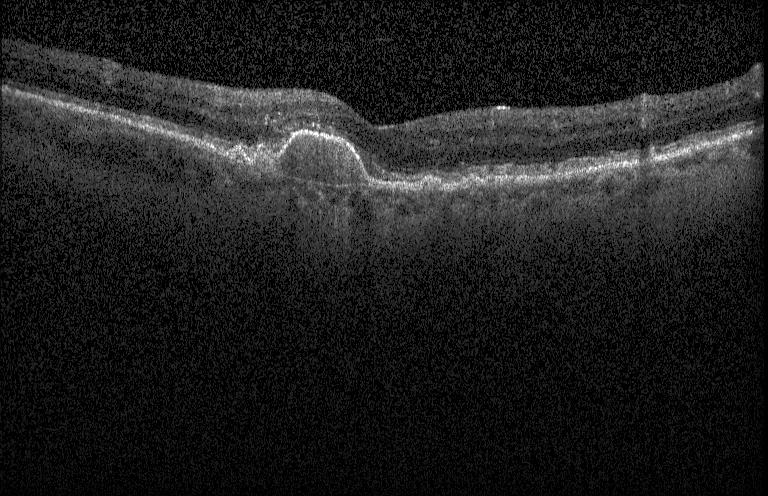
Retinal OCT cross-section; acquired on a Heidelberg Spectralis; SD-OCT; fovea-centered. This B-scan demonstrates a choroidal neovascular membrane.